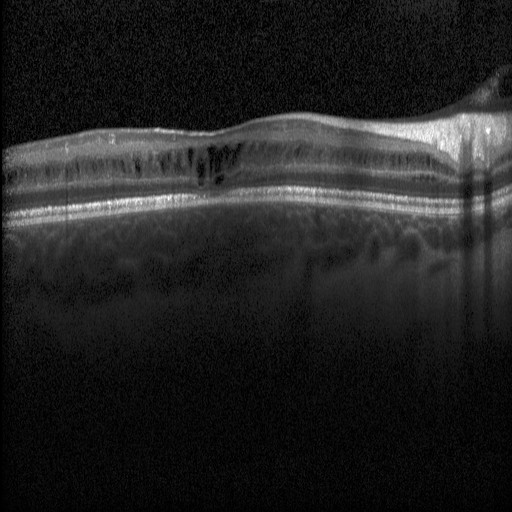 SD-OCT, acquired on a Heidelberg Spectralis, optical coherence tomography B-scan — Assessment: DME.